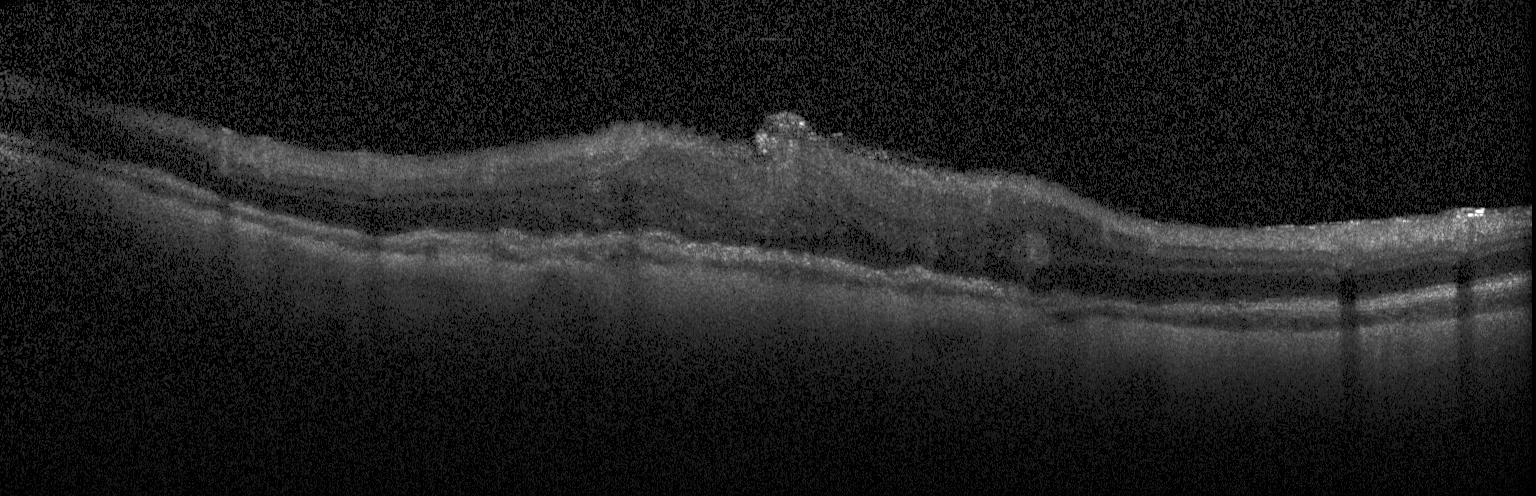
OCT B-scan, Heidelberg Spectralis OCT system.
Finding: diabetic macular edema.